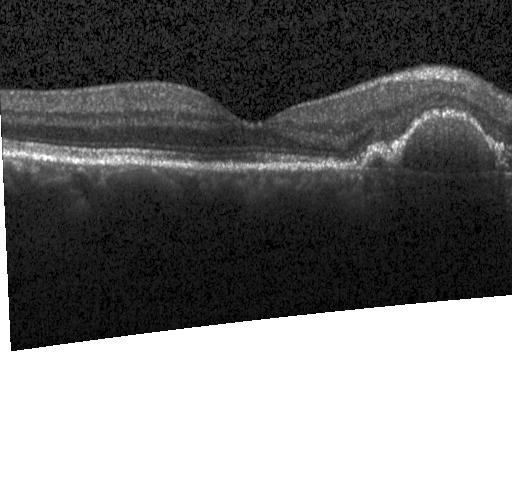 OCT finding: CNV.